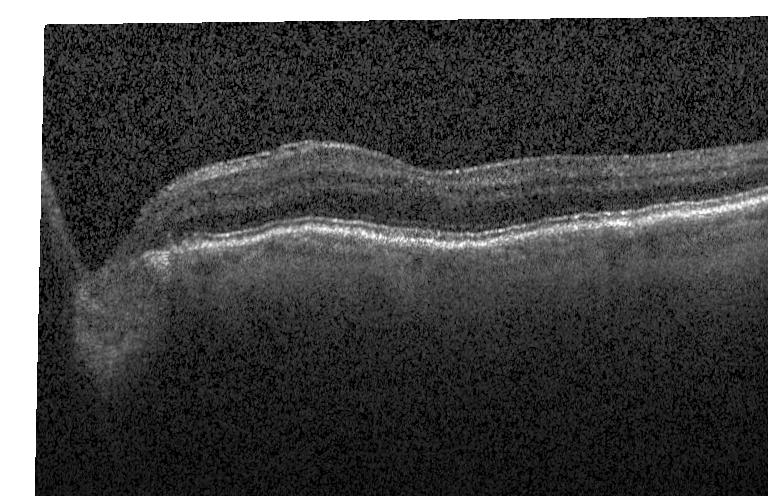 Optical coherence tomography B-scan — Finding: no choroidal neovascularization, no diabetic macular edema, and no drusen.